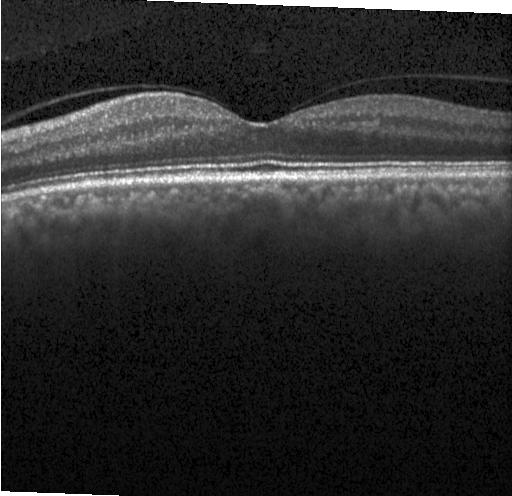

OCT finding: neither choroidal neovascularization, diabetic macular edema, nor drusen.